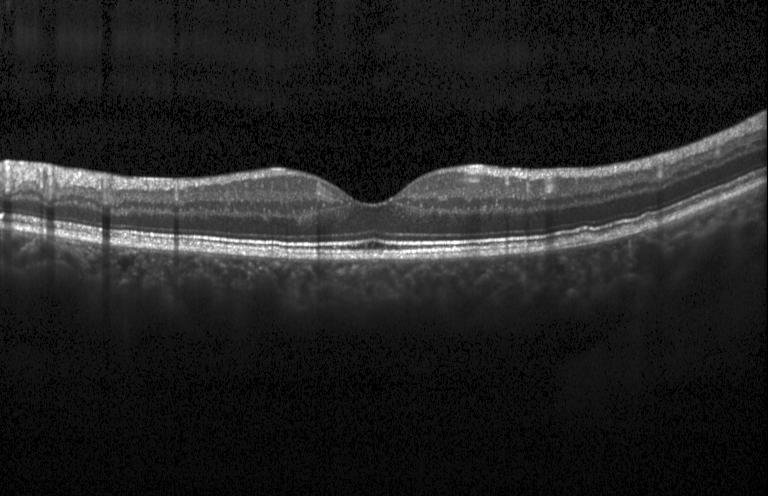 Finding: multiple drusen.